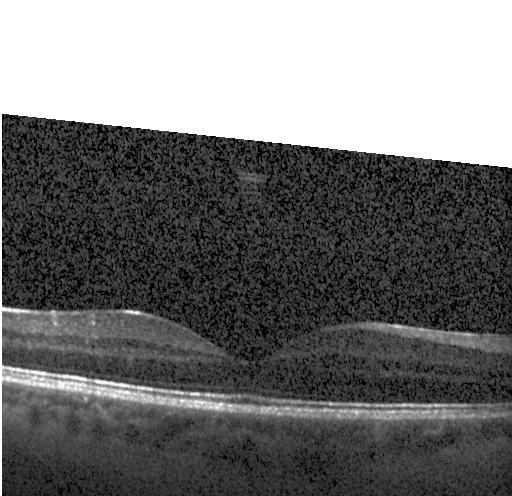 Macular scan. Spectral-domain OCT. OCT line scan.
Finding: neither choroidal neovascularization, diabetic macular edema, nor drusen.